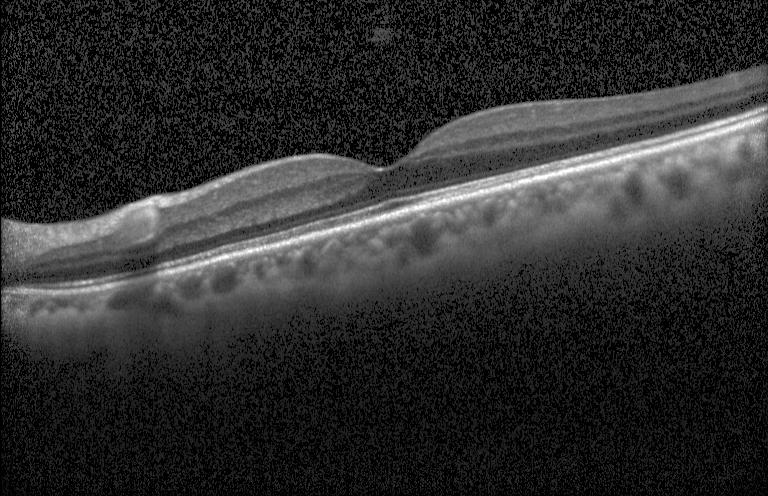

Finding: no choroidal neovascularization, no diabetic macular edema, and no drusen.